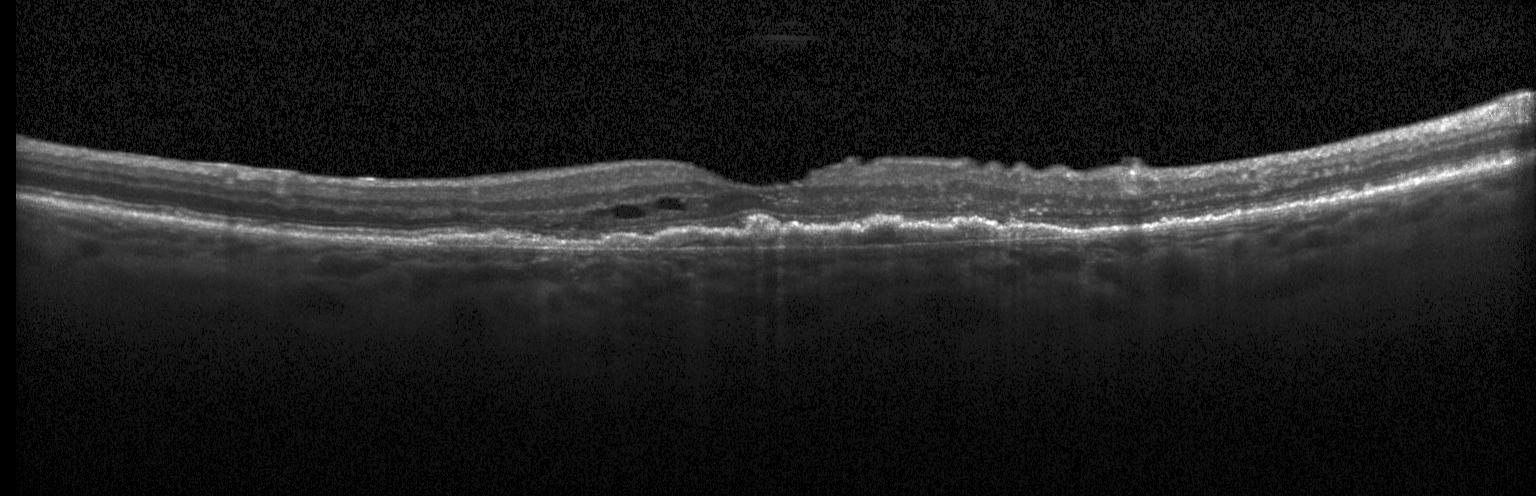
OCT B-scan showing a choroidal neovascular membrane.